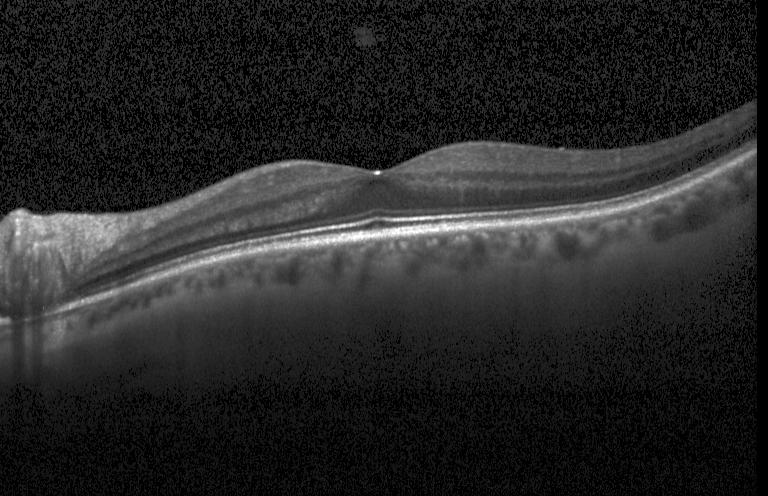
Macular OCT demonstrating no evidence of choroidal neovascularization, diabetic macular edema, or drusen.